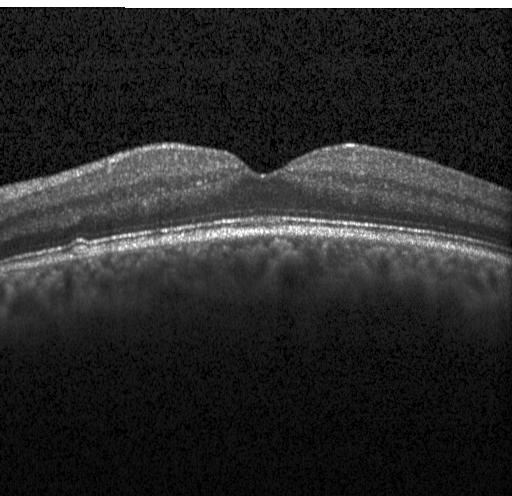

Impression: no CNV, no DME, and no drusen.